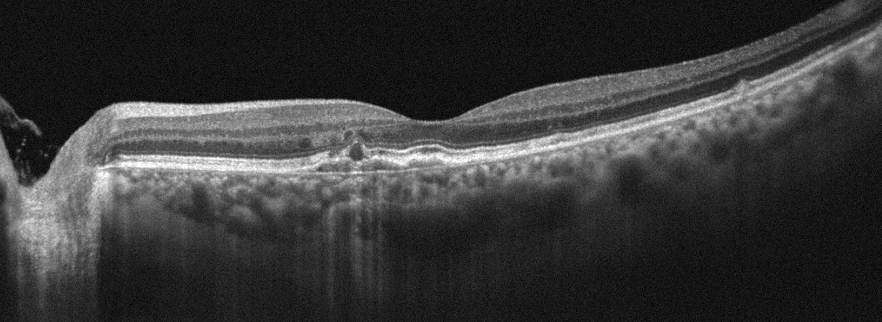
OCT scan showing age-related macular degeneration.